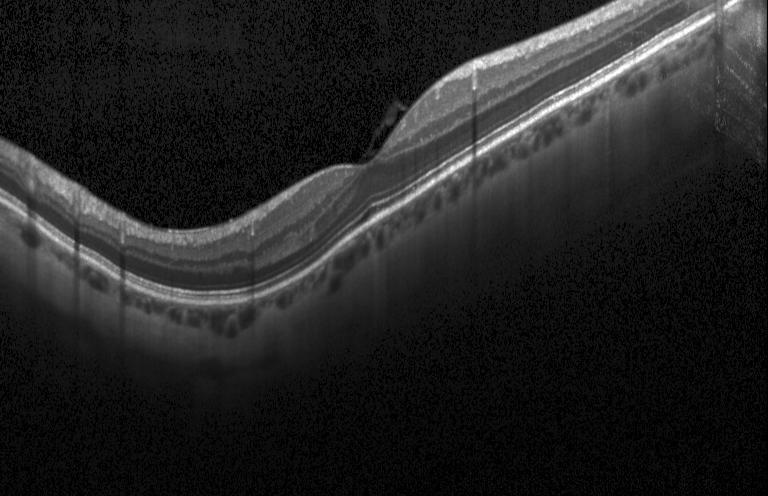
Macular scan, retinal OCT B-scan, Heidelberg Spectralis
Finding: no CNV, no DME, and no drusen.